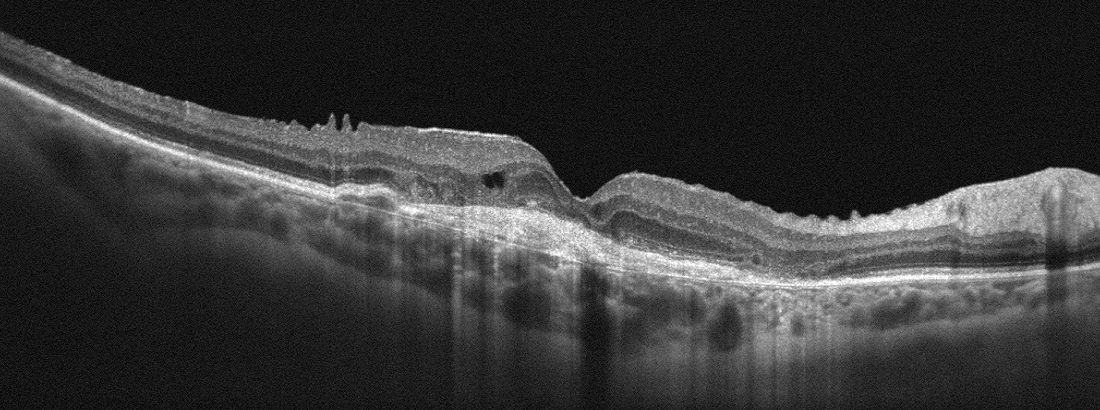

Fovea-centered. Optical coherence tomography B-scan. Diagnosis: AMD.